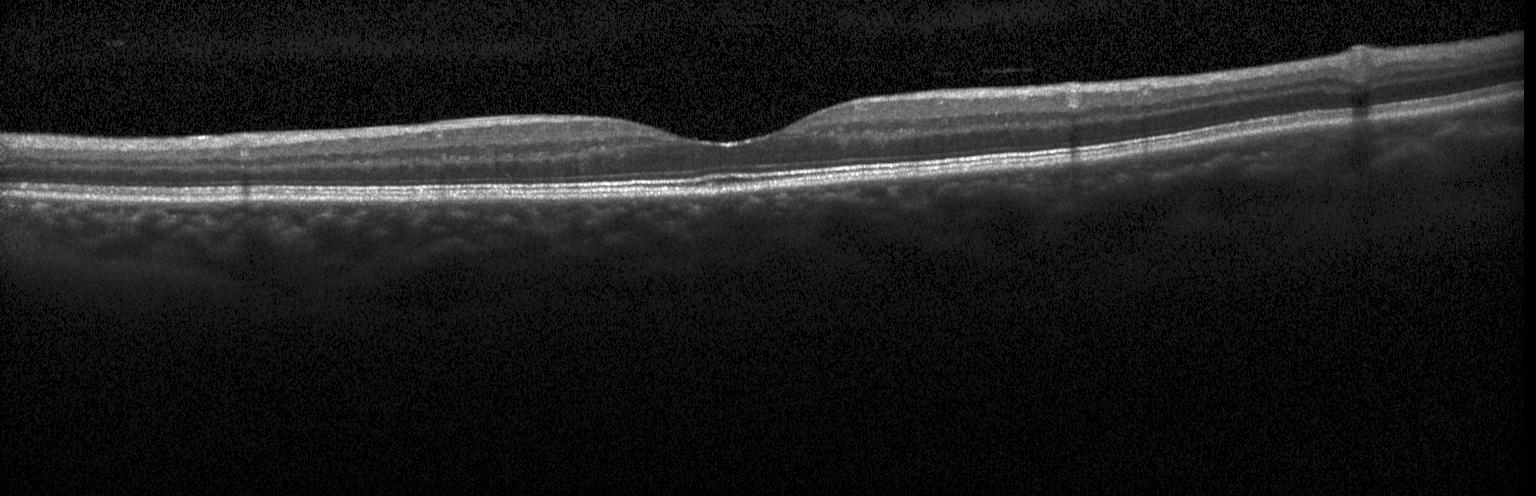
Retinal OCT B-scan.
The scan shows no evidence of choroidal neovascularization, diabetic macular edema, or drusen.